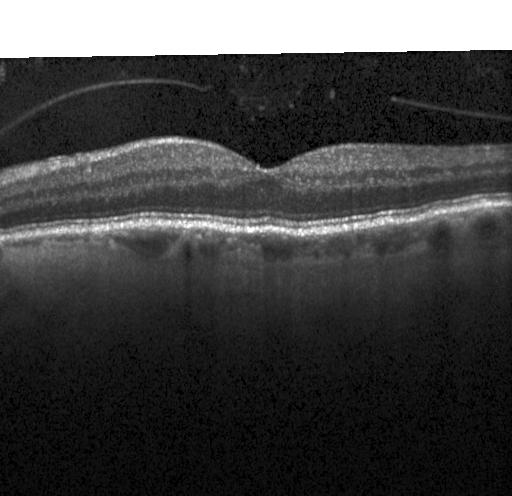 Dx: neither choroidal neovascularization, diabetic macular edema, nor drusen.